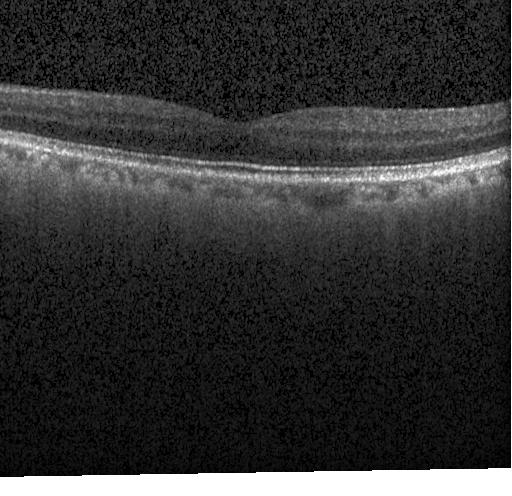

Retinal OCT cross-section, acquired on a Heidelberg Spectralis, through the macula, spectral-domain optical coherence tomography.
No evidence of CNV, DME, or drusen.